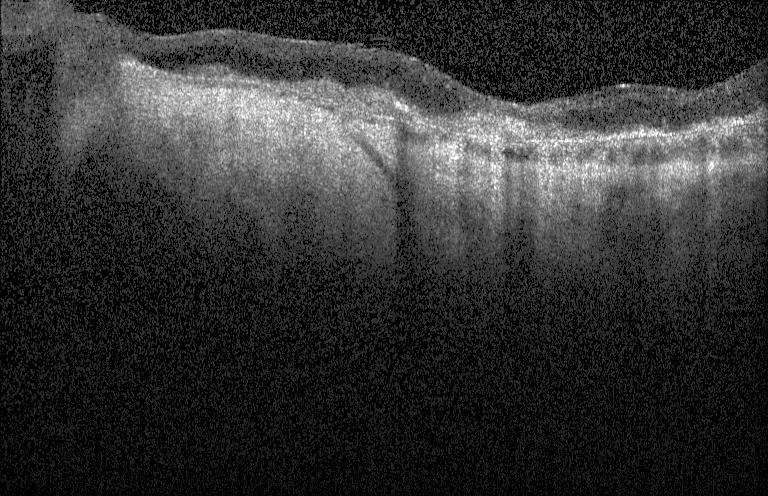

Through the macula; acquired on a Heidelberg Spectralis; OCT line scan — Finding: a choroidal neovascular membrane.